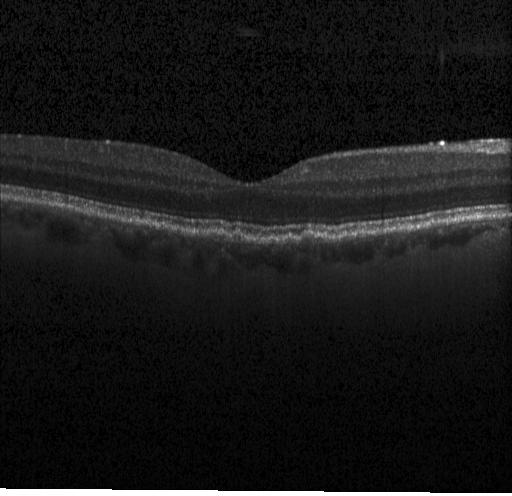
Instrument: Heidelberg Spectralis, spectral-domain OCT, retinal OCT B-scan.
Diagnosis: multiple drusen.